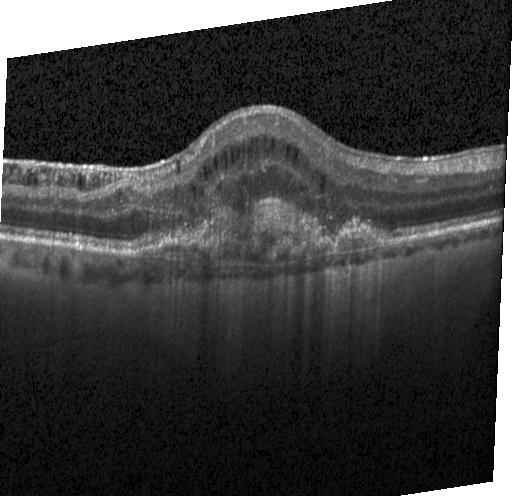

Optical coherence tomography B-scan.
Finding: choroidal neovascularization (CNV).